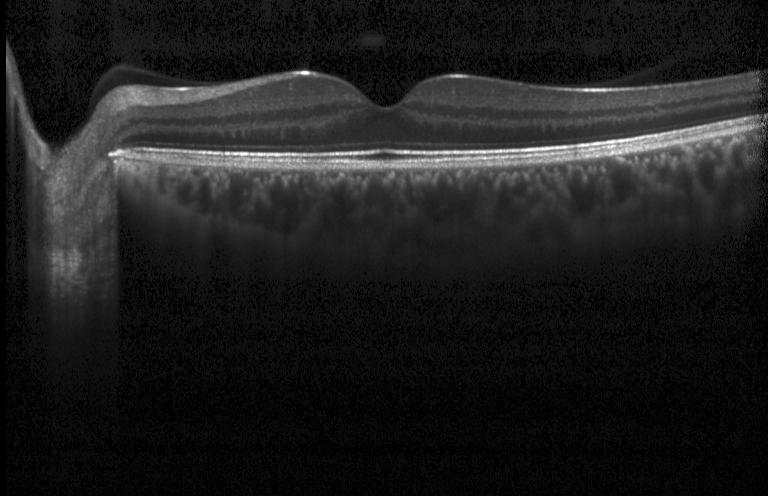 Retinal OCT B-scan, Heidelberg Spectralis OCT system, macular scan. Diagnosis: no choroidal neovascularization, diabetic macular edema, or drusen.